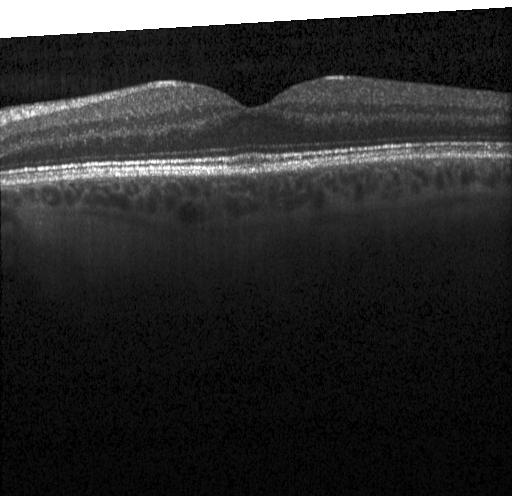

OCT line scan · acquired on a Heidelberg Spectralis — OCT finding: no choroidal neovascularization, no diabetic macular edema, and no drusen.